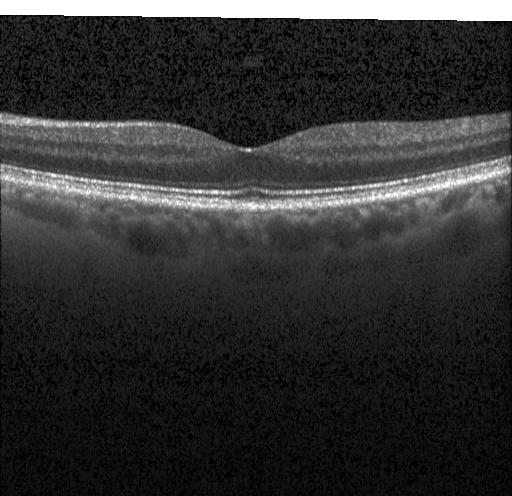 Impression: no CNV, DME, or drusen.